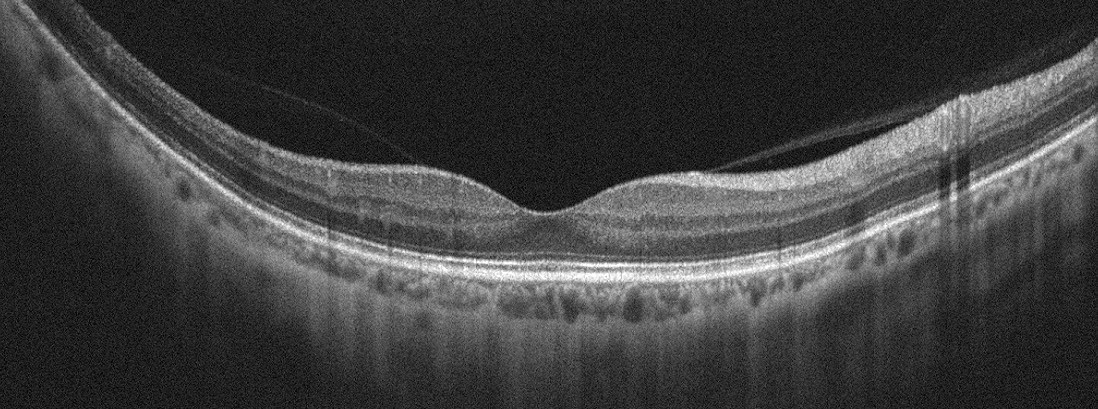
Macular OCT: no evidence of AMD, DME, ERM, RAO, RVO, or VID.